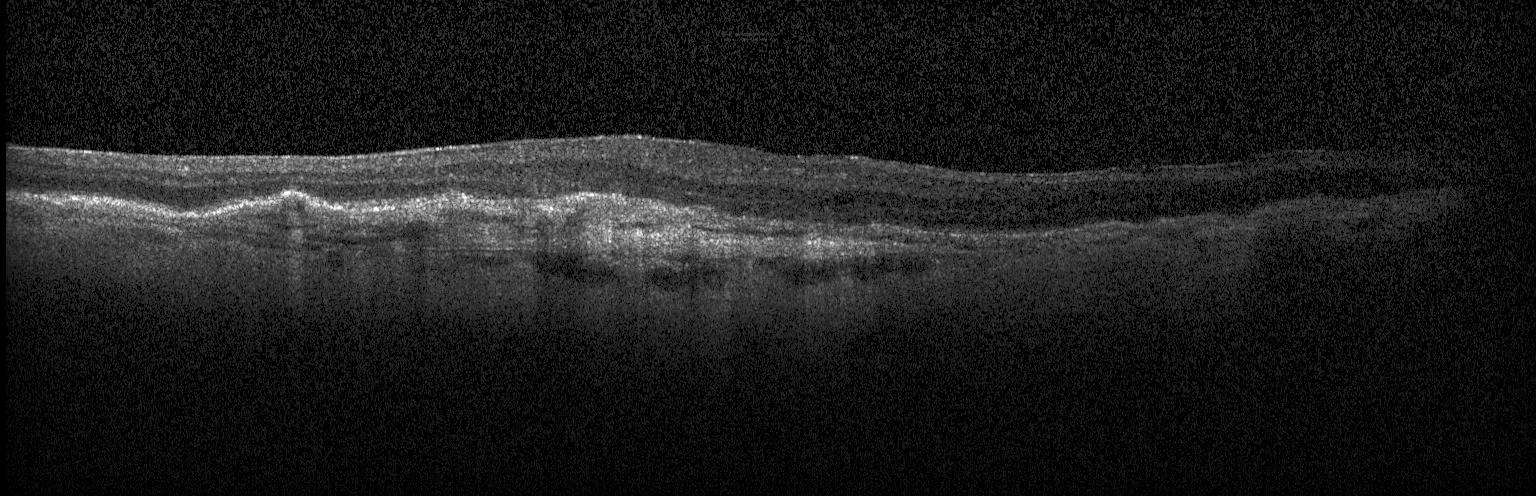
Macular OCT demonstrating choroidal neovascularization.